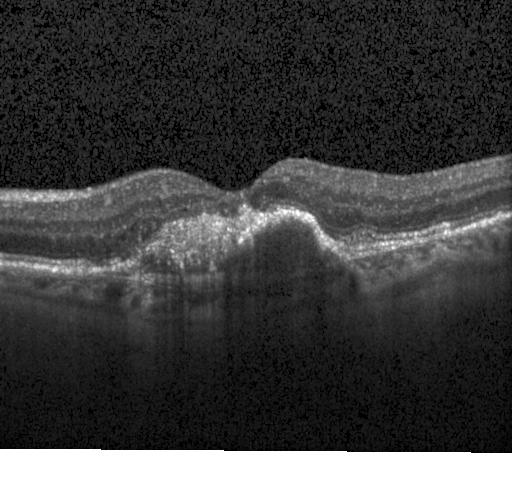
Heidelberg Spectralis; centered on the fovea; OCT line scan. Impression: CNV.